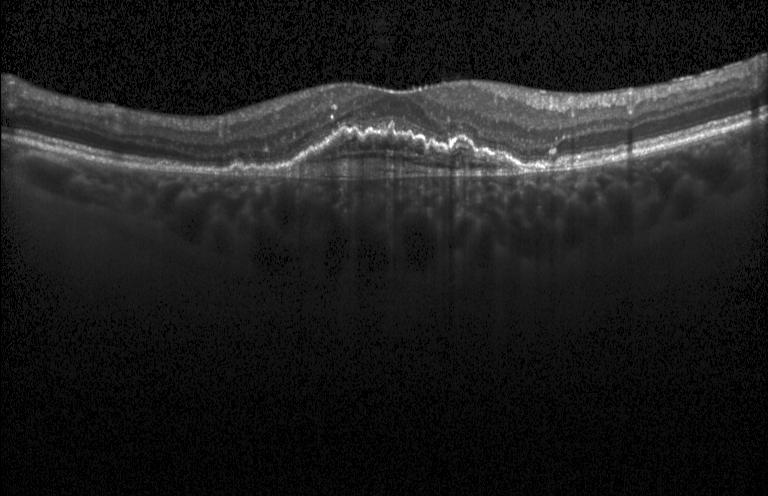

Centered on the fovea · retinal OCT cross-section · Heidelberg Spectralis. Diagnosis: choroidal neovascularization (CNV).